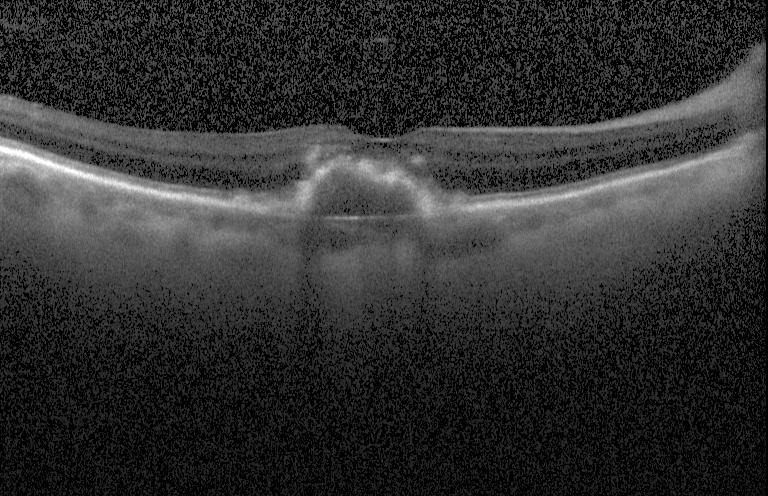

Spectral-domain OCT · centered on the fovea · optical coherence tomography B-scan · Heidelberg Spectralis OCT system
CNV.